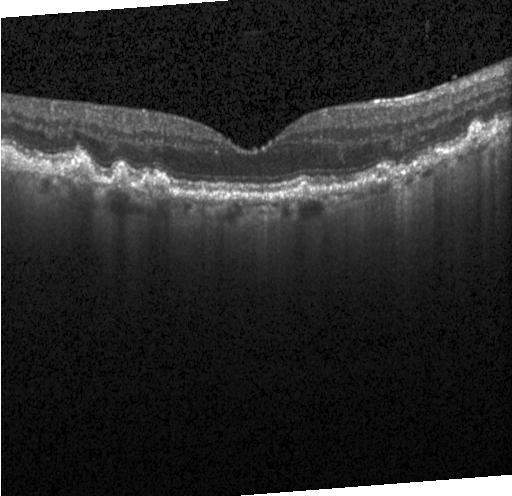

Retinal OCT B-scan
Finding: drusen.